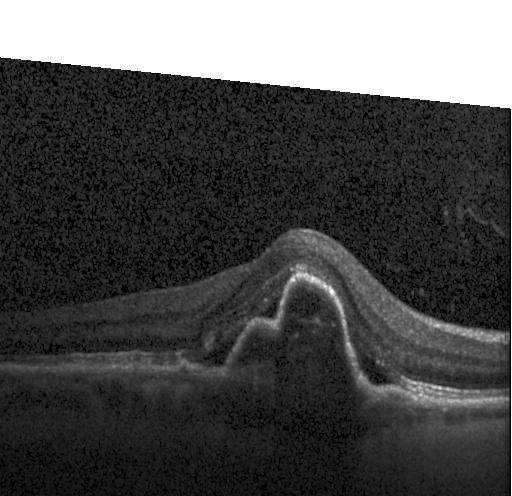 OCT scan showing a choroidal neovascular membrane.